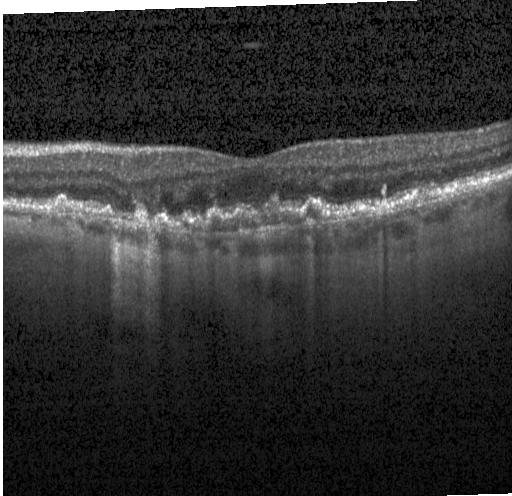 Retinal OCT cross-section. Horizontal scan through the fovea.
Diagnosis: choroidal neovascularization (CNV).